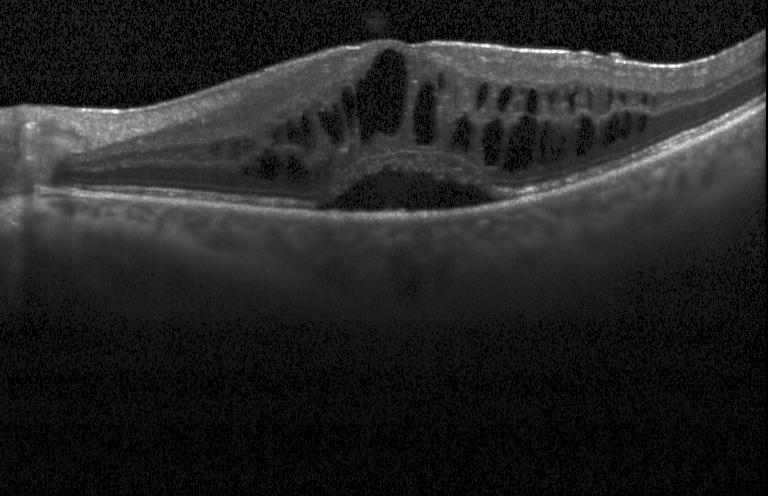

OCT B-scan. Diagnosis: DME.